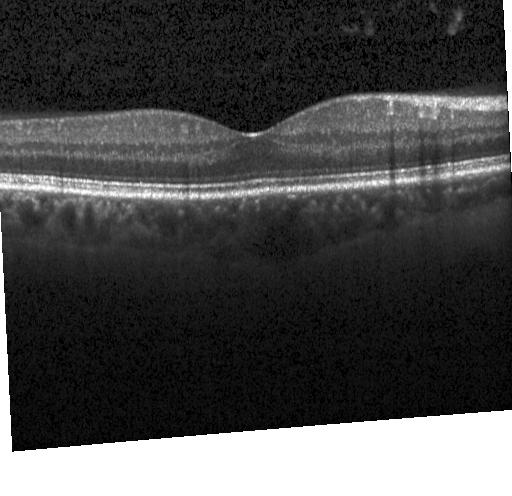 Optical coherence tomography B-scan, horizontal scan through the fovea, spectral-domain OCT.
Impression: neither choroidal neovascularization, diabetic macular edema, nor drusen.